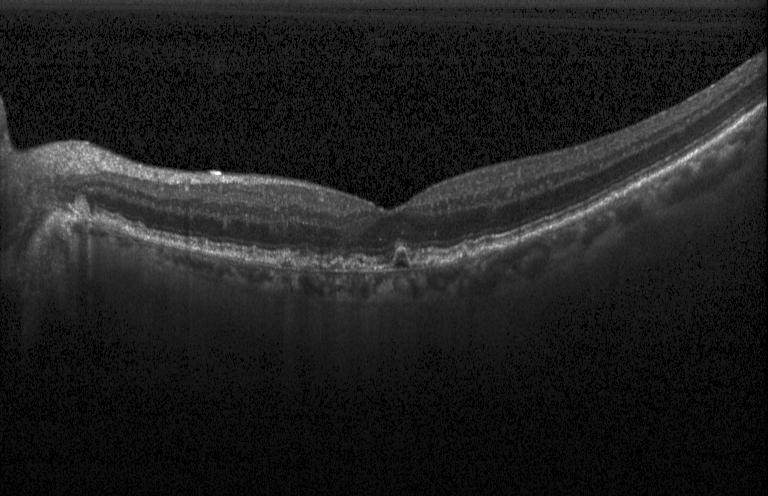

Macular scan. Retinal OCT cross-section
Macular OCT: CNV.